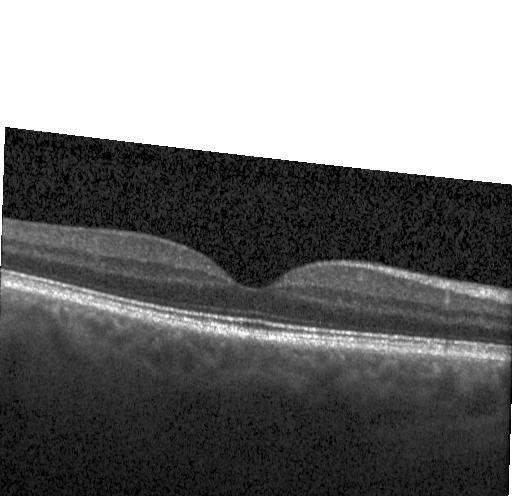 No evidence of choroidal neovascularization, diabetic macular edema, or drusen.